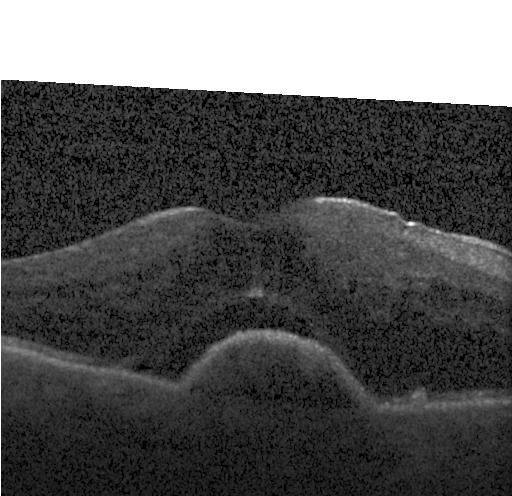 Impression: CNV.